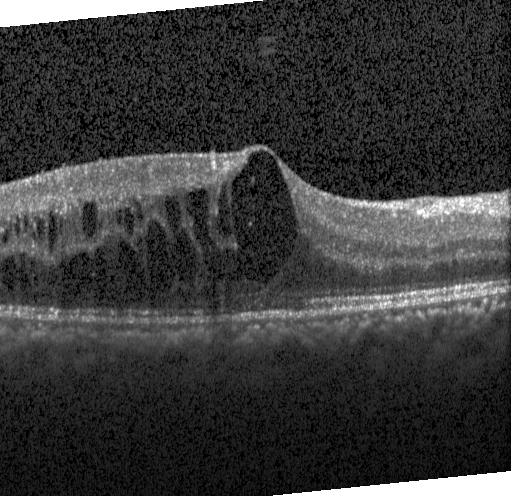 OCT scan showing diabetic macular edema.